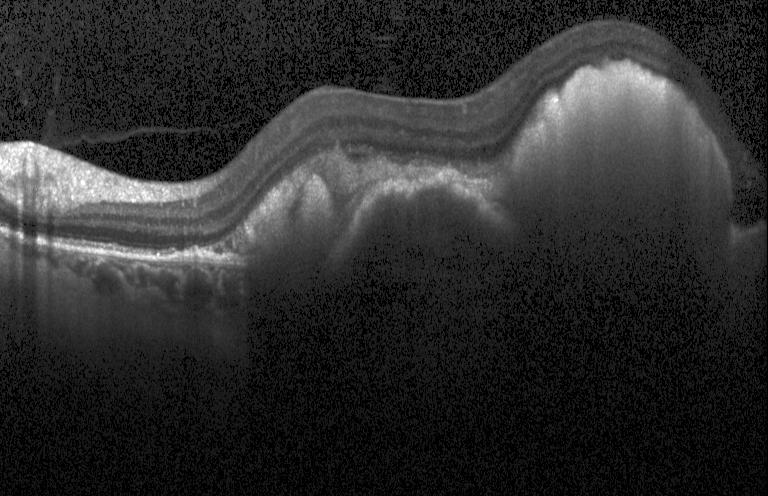
Impression: a choroidal neovascular membrane.